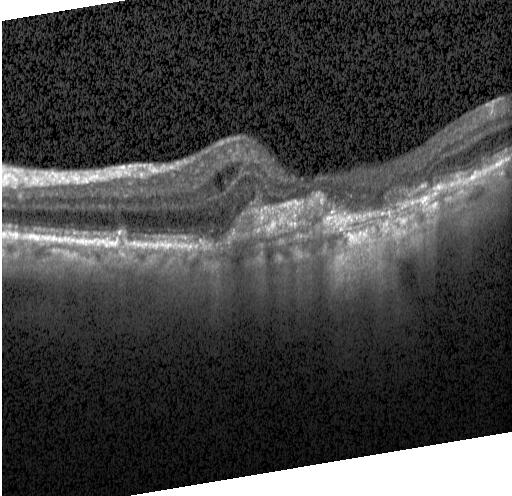
Diagnosis: a choroidal neovascular membrane.